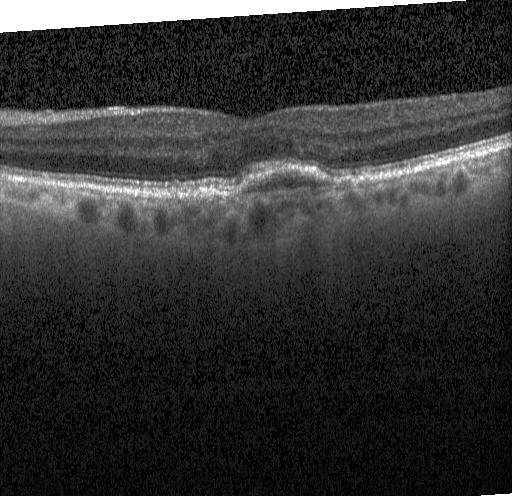

Impression: a choroidal neovascular membrane.